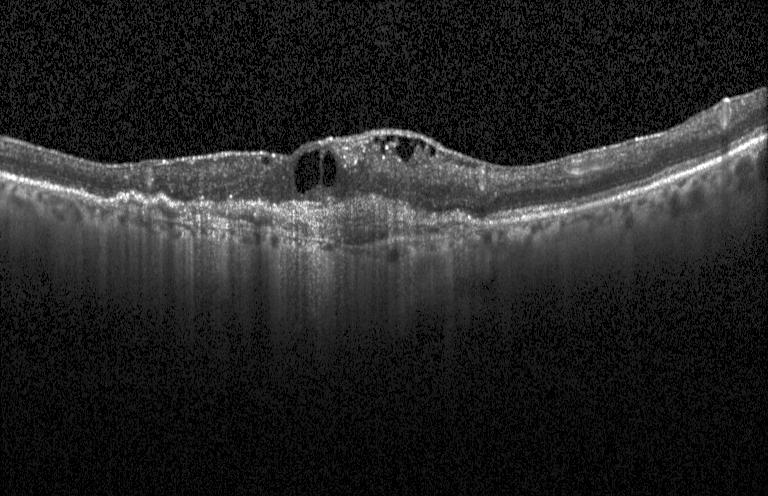

OCT finding: a choroidal neovascular membrane.